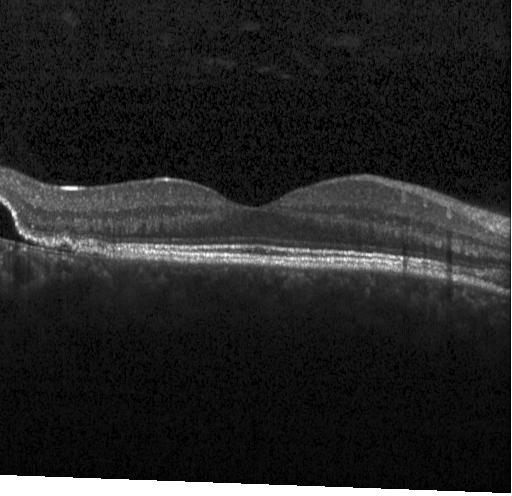

This B-scan demonstrates choroidal neovascularization (CNV).